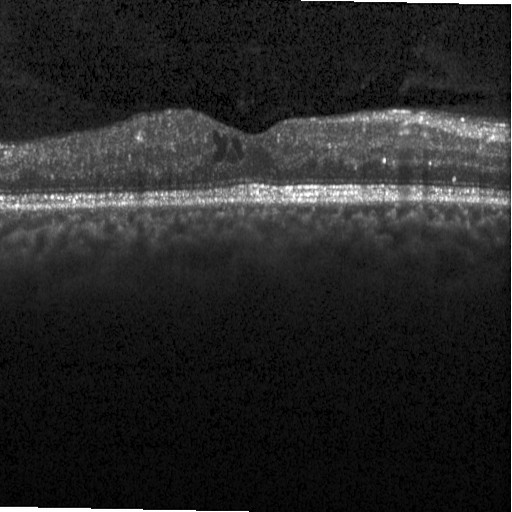
Impression: diabetic macular edema (DME).